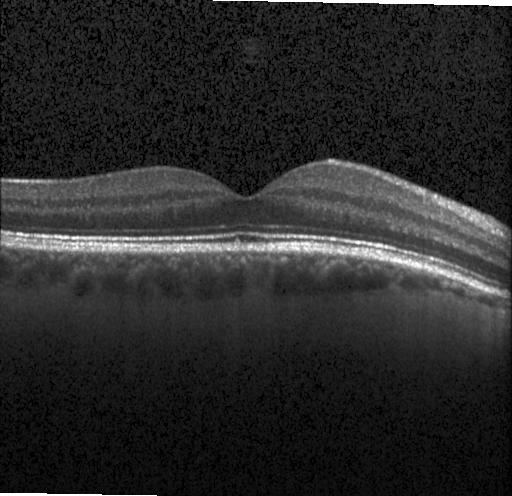

OCT line scan
Finding: no choroidal neovascularization, no diabetic macular edema, and no drusen.